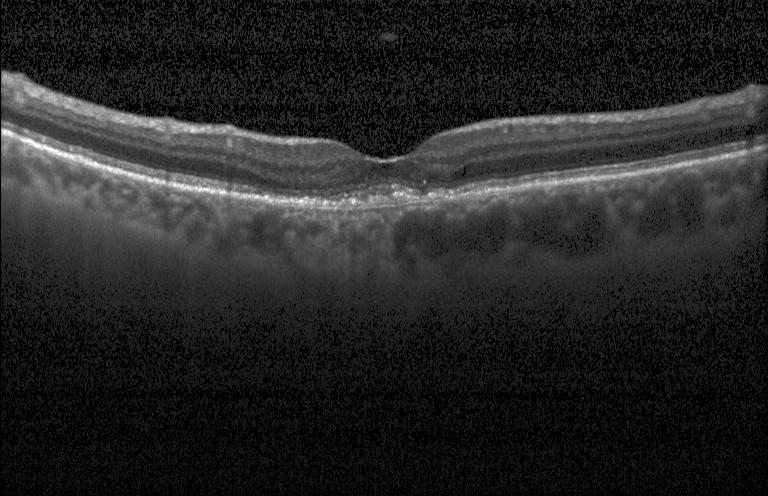 OCT scan showing choroidal neovascularization (CNV).